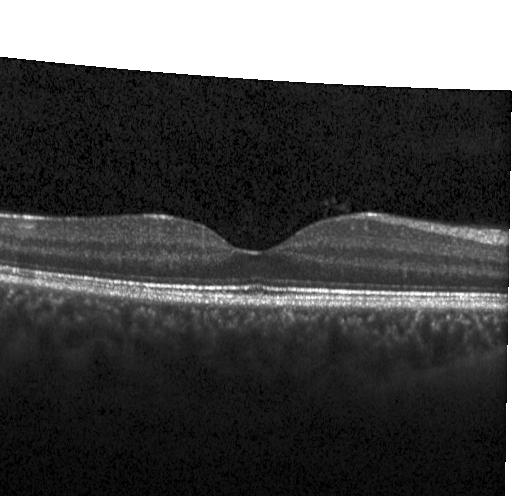

Spectral-domain optical coherence tomography. Optical coherence tomography B-scan
Diagnosis: no evidence of choroidal neovascularization, diabetic macular edema, or drusen.